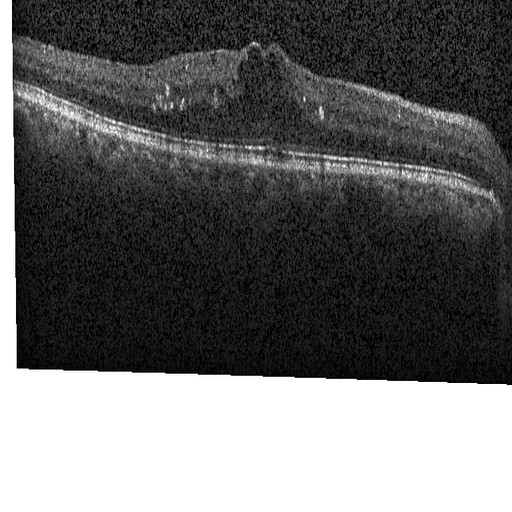
Spectral-domain OCT; Heidelberg Spectralis; retinal OCT B-scan; macular scan
Diabetic macular edema (DME).